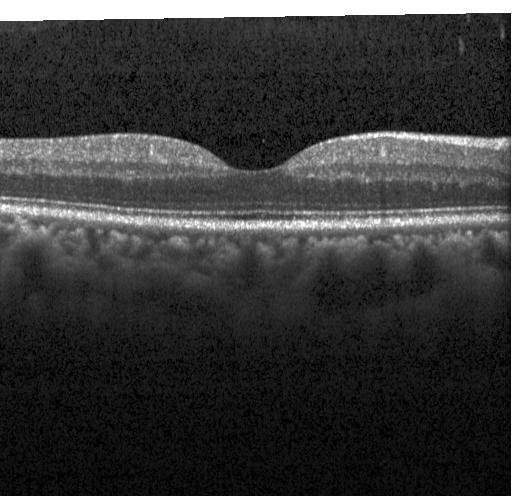
Retinal OCT B-scan · Heidelberg Spectralis.
The scan shows neither choroidal neovascularization, diabetic macular edema, nor drusen.